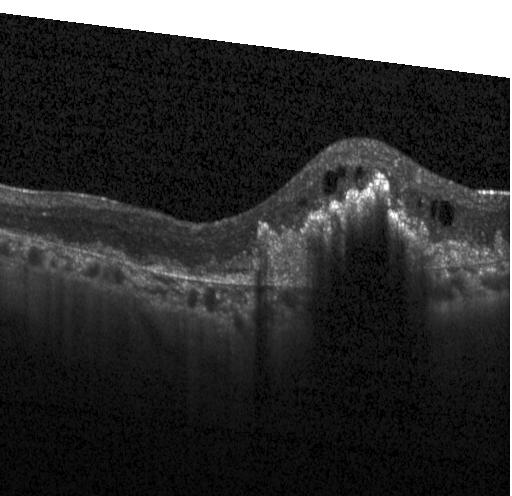
This B-scan demonstrates a choroidal neovascular membrane.